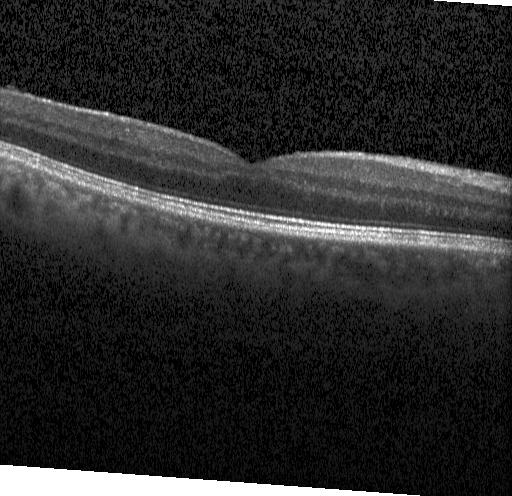

The scan shows no evidence of CNV, DME, or drusen.